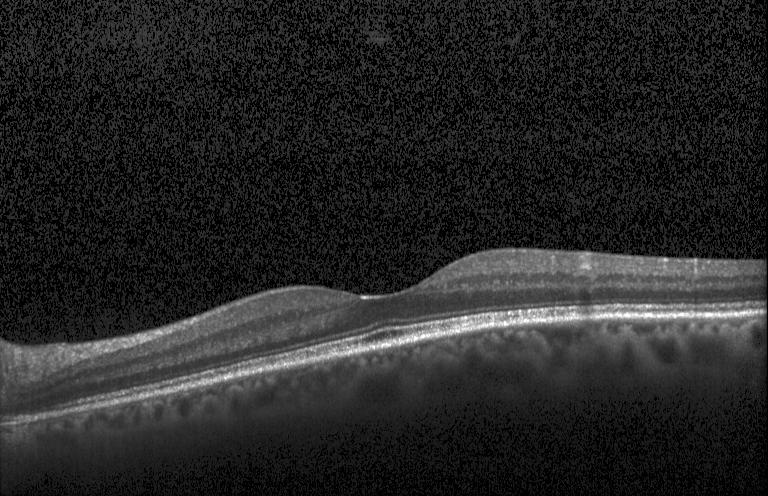
Optical coherence tomography scan
Dx: no choroidal neovascularization, no diabetic macular edema, and no drusen.